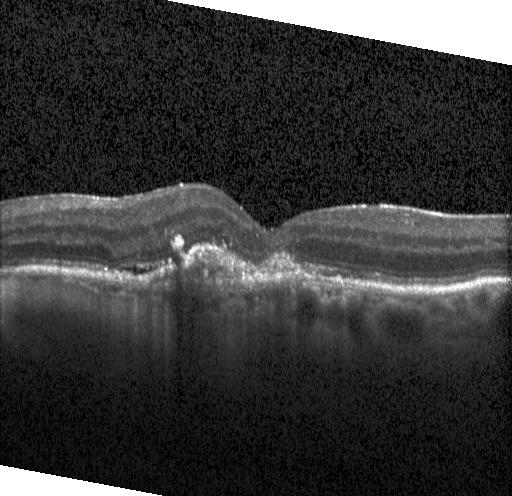
Heidelberg Spectralis · retinal OCT cross-section · centered on the fovea · spectral-domain OCT. Diagnosis: a choroidal neovascular membrane.